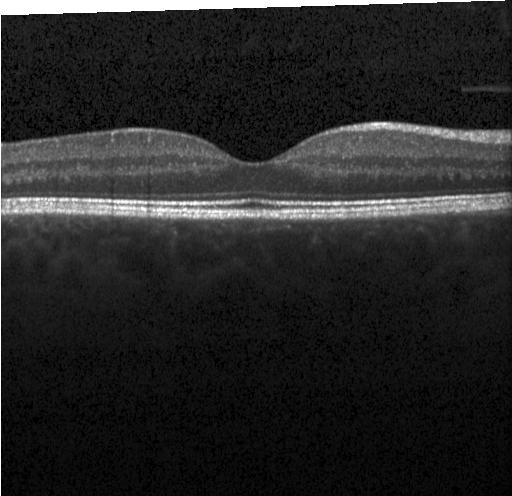 Impression: no choroidal neovascularization, diabetic macular edema, or drusen.